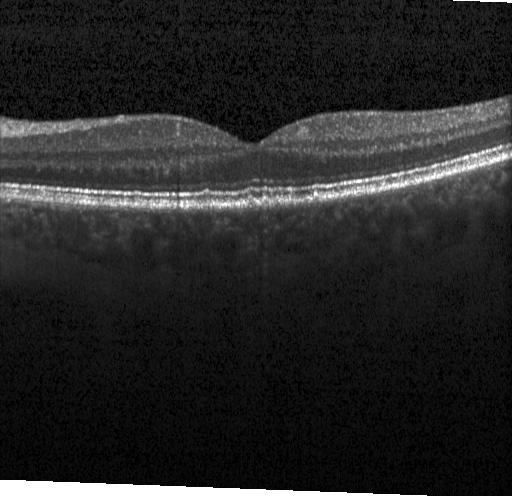

OCT line scan
Impression: multiple drusen.